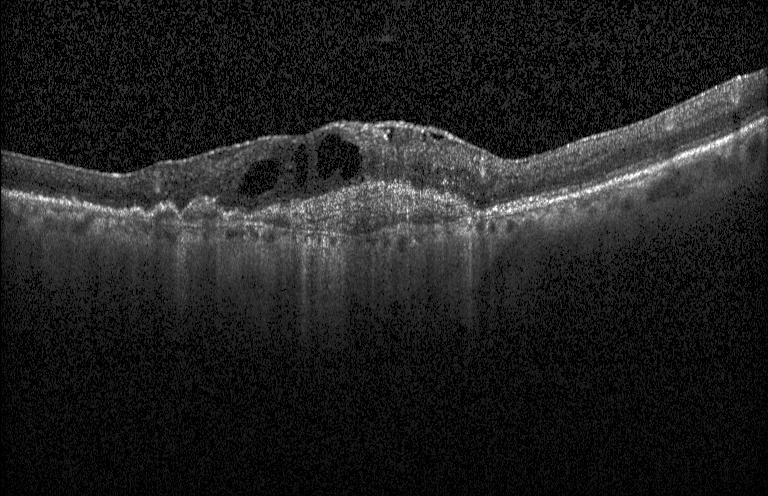

Retinal OCT cross-section
Finding: a choroidal neovascular membrane.